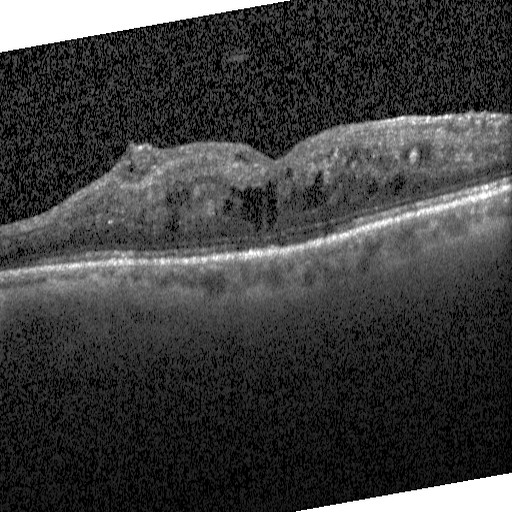

OCT finding: diabetic macular edema (DME).